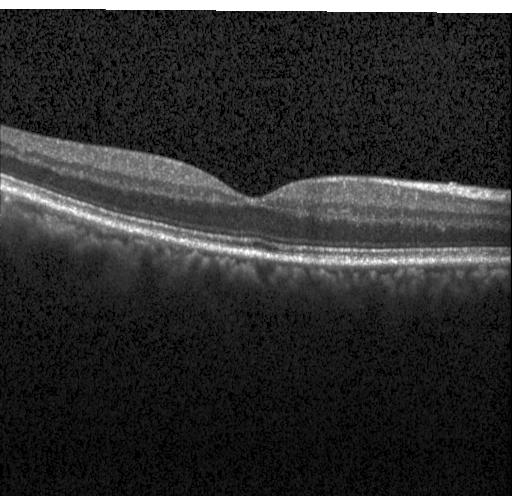 Impression: no CNV, no DME, and no drusen.